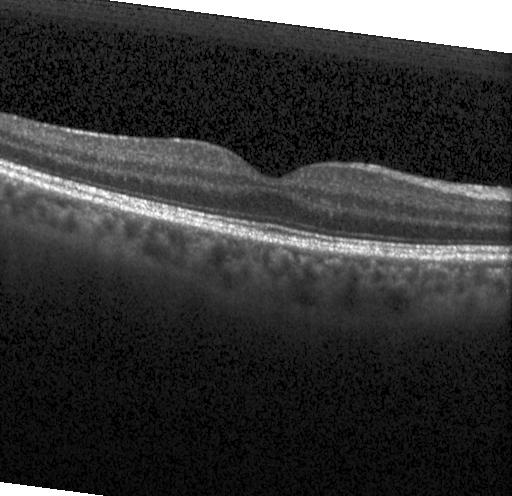

Macular OCT: no evidence of CNV, DME, or drusen.